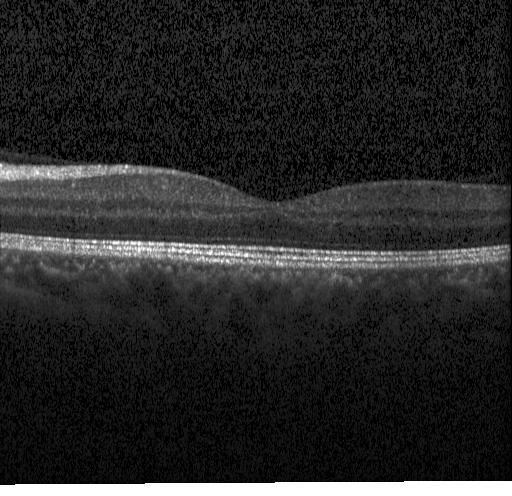
Retinal OCT cross-section showing neither choroidal neovascularization, diabetic macular edema, nor drusen.